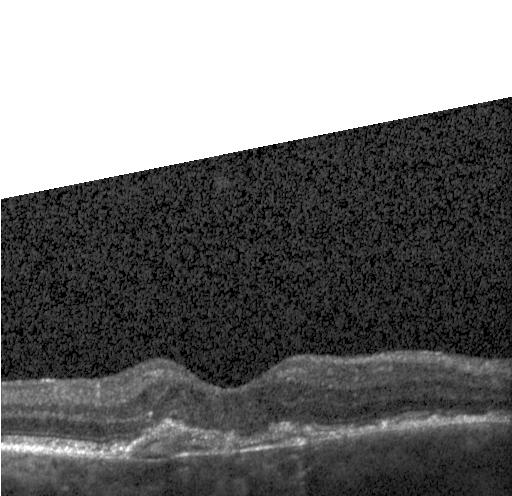
Spectral-domain optical coherence tomography, retinal OCT cross-section, macular scan, instrument: Heidelberg Spectralis — Assessment: a choroidal neovascular membrane.